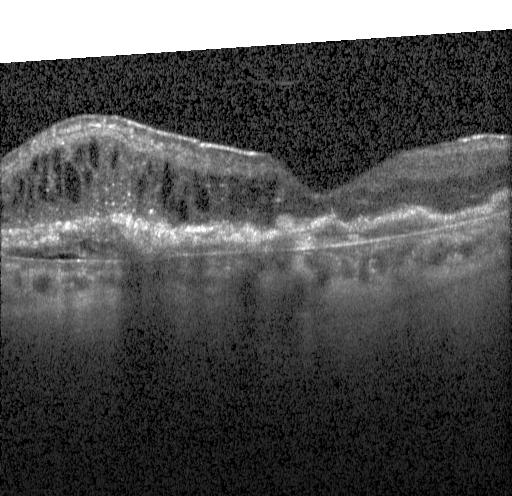
Spectral-domain optical coherence tomography. OCT line scan. Through the macula. Acquired on a Heidelberg Spectralis. Diagnosis: choroidal neovascularization.